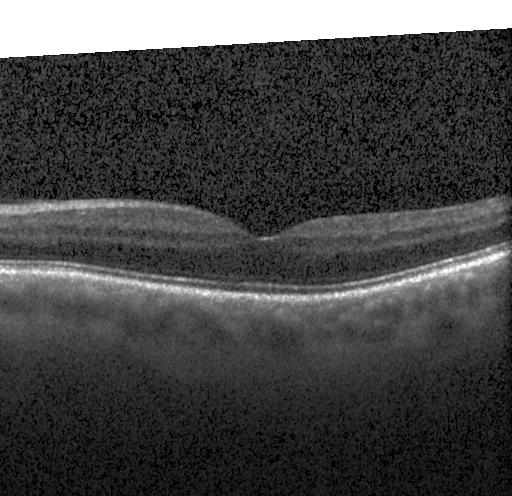 OCT scan showing no CNV, DME, or drusen.